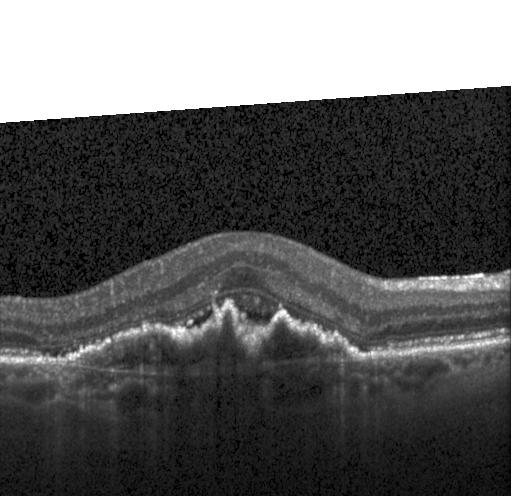

OCT line scan · spectral-domain optical coherence tomography. Macular OCT: a choroidal neovascular membrane.